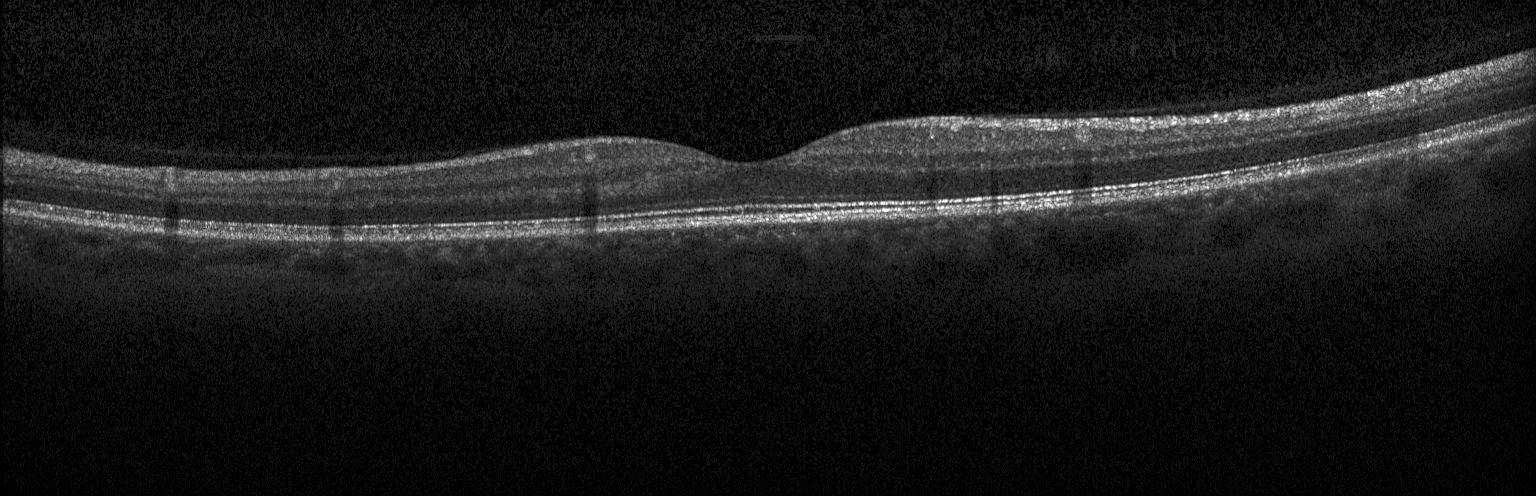
Optical coherence tomography scan; spectral-domain optical coherence tomography
Dx: neither CNV, DME, nor drusen.